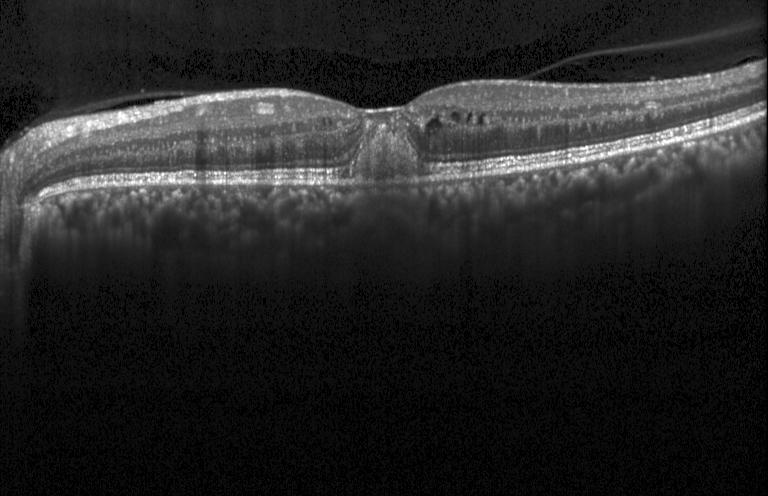
SD-OCT. Instrument: Heidelberg Spectralis. Fovea-centered. Optical coherence tomography B-scan.
Assessment: a choroidal neovascular membrane.